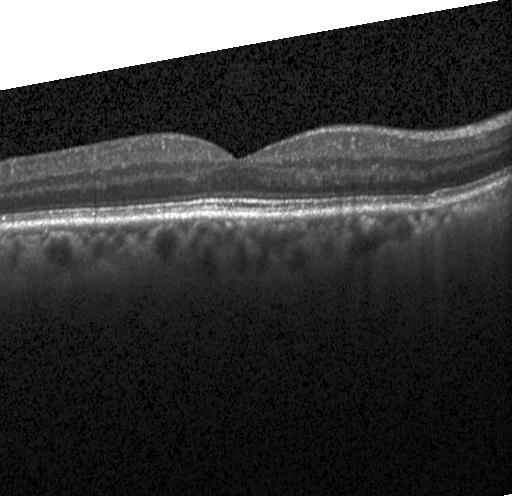

Optical coherence tomography scan, horizontal scan through the fovea, spectral-domain OCT, instrument: Heidelberg Spectralis — Impression: no evidence of choroidal neovascularization, diabetic macular edema, or drusen.